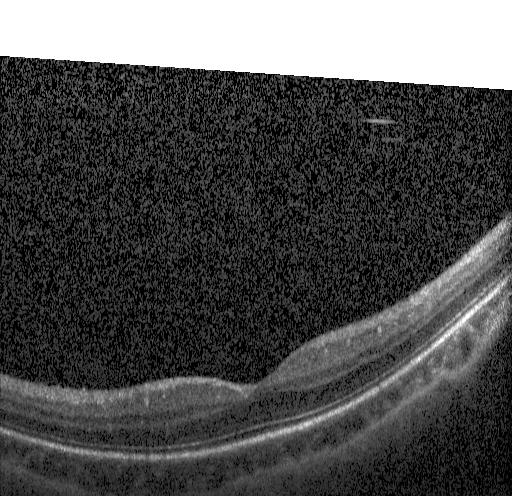 Spectral-domain optical coherence tomography; OCT line scan; through the macula; Heidelberg Spectralis OCT system — This B-scan demonstrates no CNV, DME, or drusen.